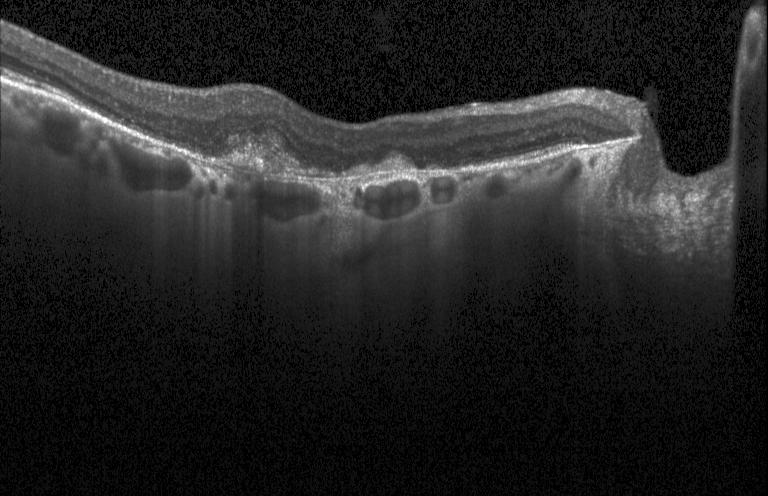 Macular scan, OCT B-scan, acquired on a Heidelberg Spectralis — Impression: a choroidal neovascular membrane.